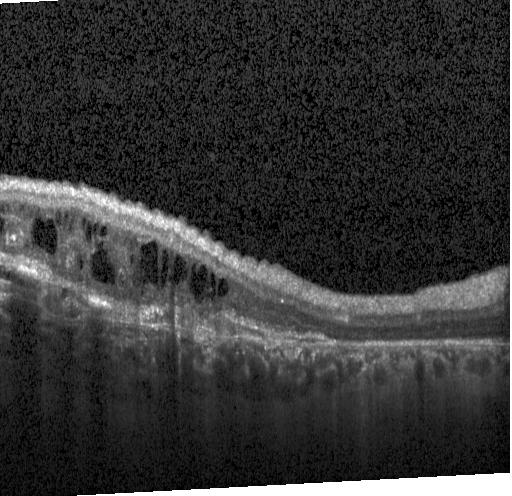
OCT line scan; Heidelberg Spectralis
Impression: a choroidal neovascular membrane.